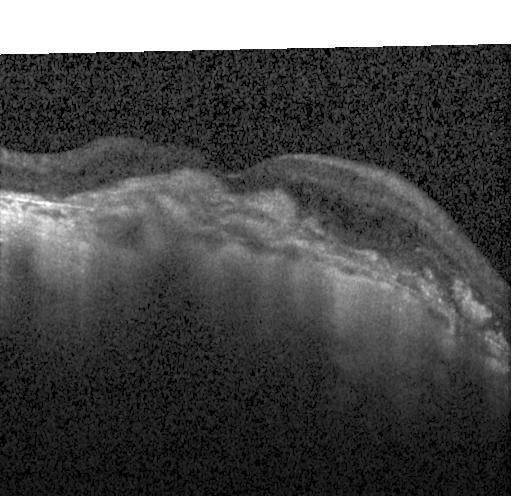 Optical coherence tomography B-scan.
Dx: choroidal neovascularization (CNV).